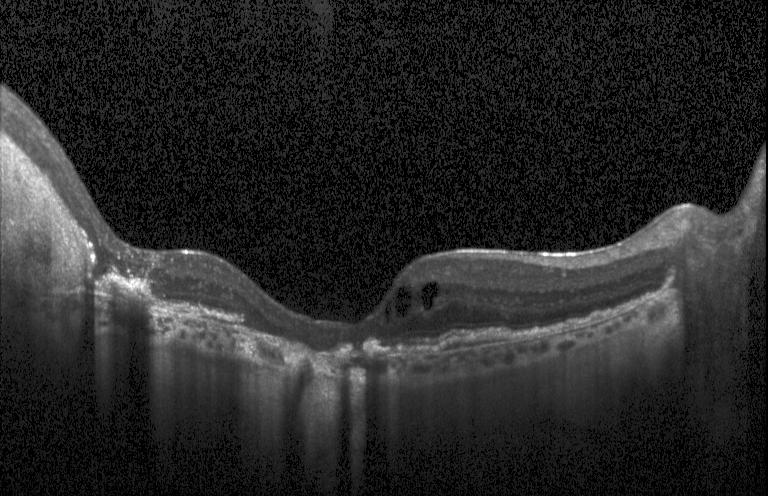 Retinal OCT B-scan.
Impression: CNV.